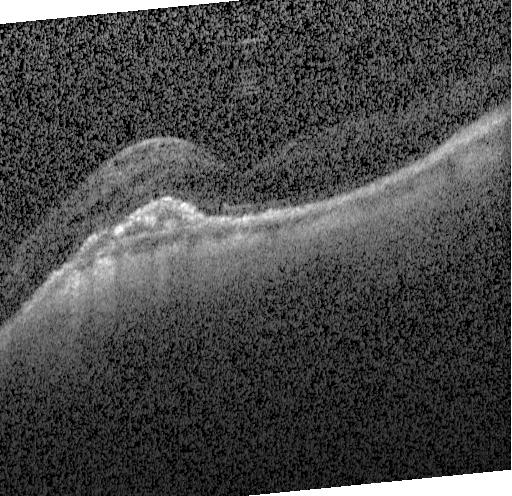 Retinal OCT B-scan. Centered on the fovea. Diagnosis: choroidal neovascularization.